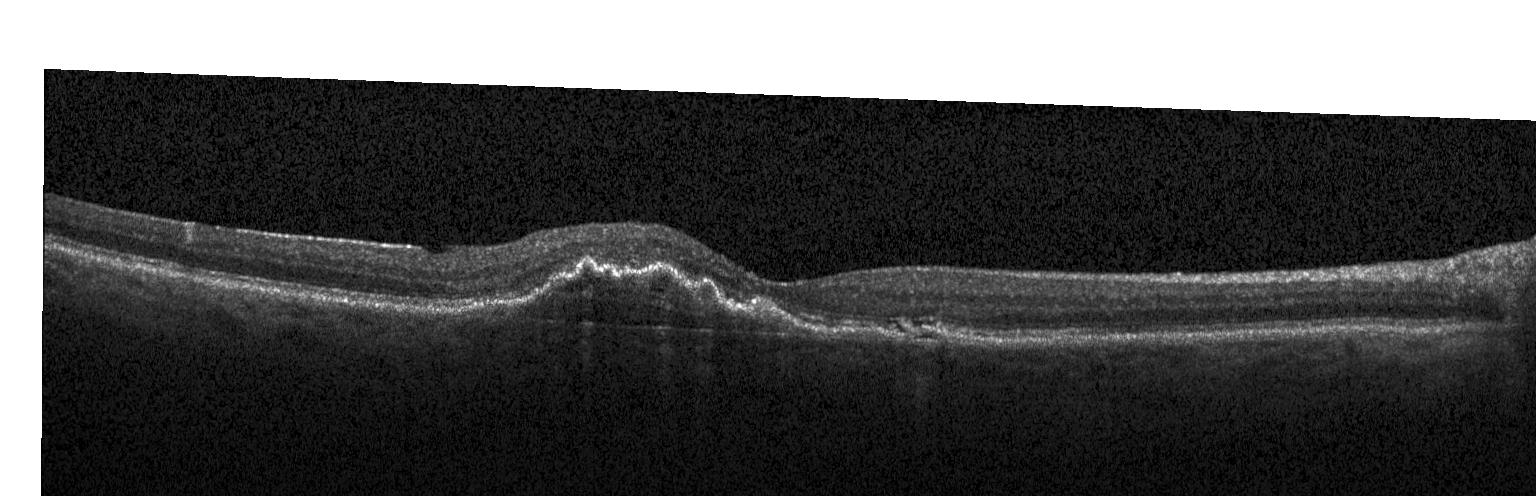
Optical coherence tomography B-scan · acquired on a Heidelberg Spectralis · fovea-centered — Impression: a choroidal neovascular membrane.